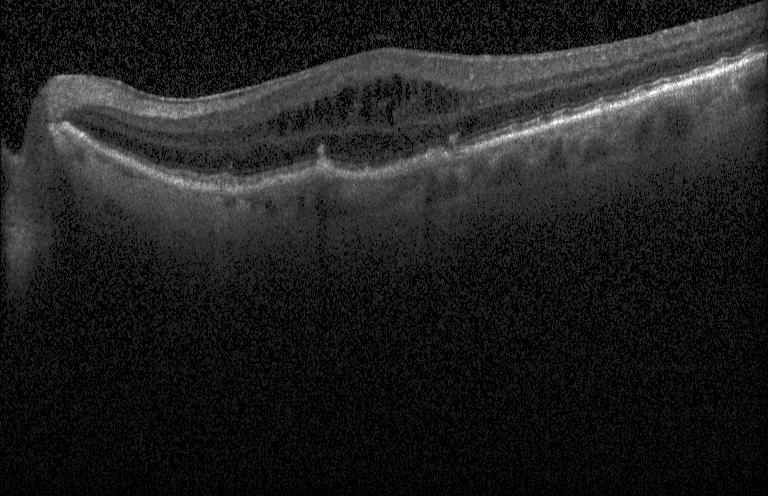 OCT line scan.
Finding: CNV.